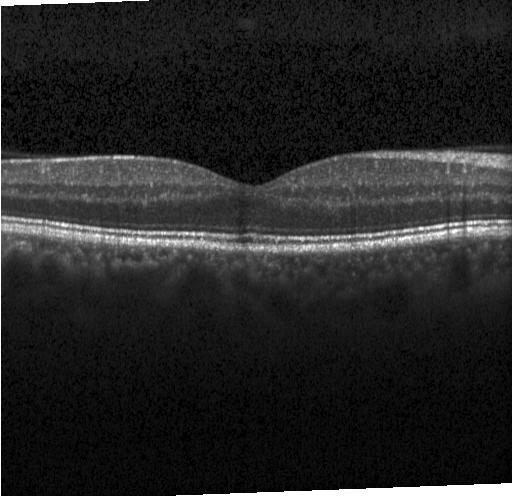 Retinal OCT cross-section; spectral-domain OCT; horizontal scan through the fovea; acquired on a Heidelberg Spectralis
Finding: no evidence of CNV, DME, or drusen.